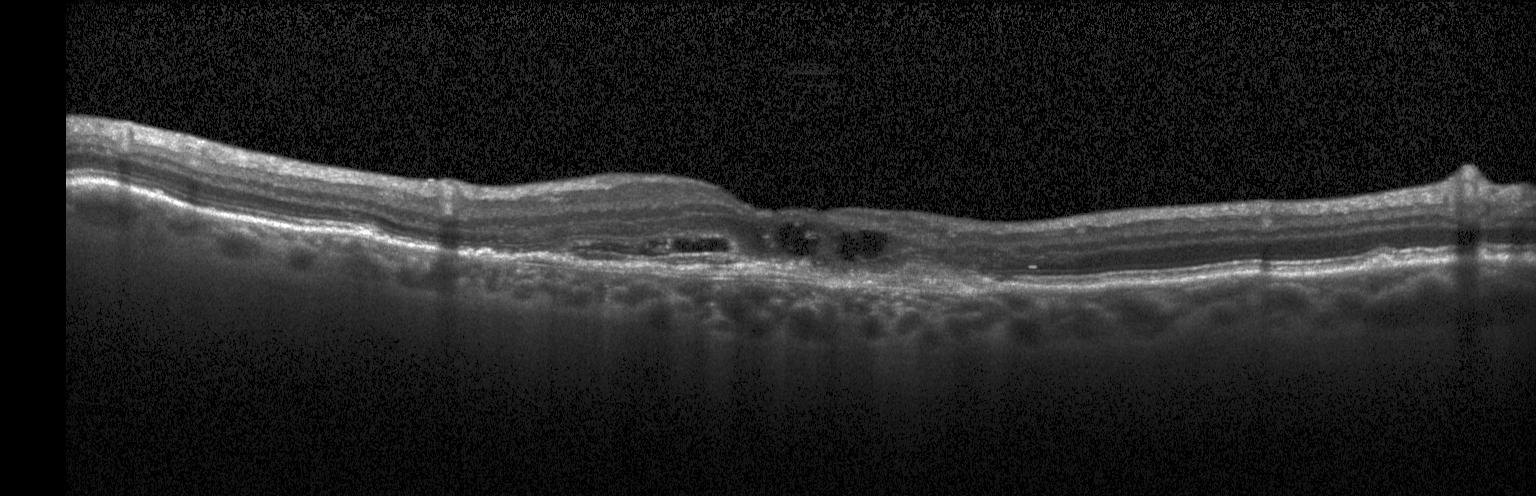

Impression: a choroidal neovascular membrane.